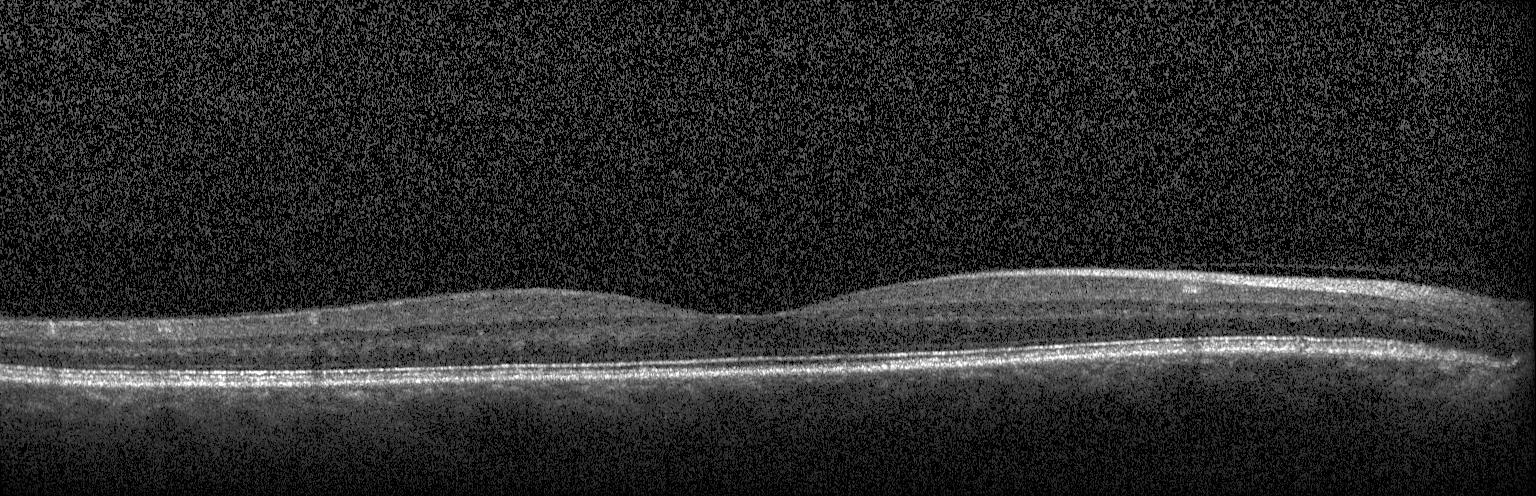 Retinal OCT B-scan
OCT finding: no choroidal neovascularization, no diabetic macular edema, and no drusen.